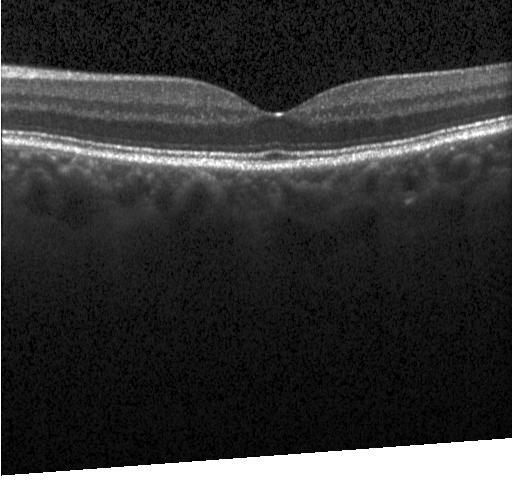 Retinal OCT cross-section showing neither choroidal neovascularization, diabetic macular edema, nor drusen.